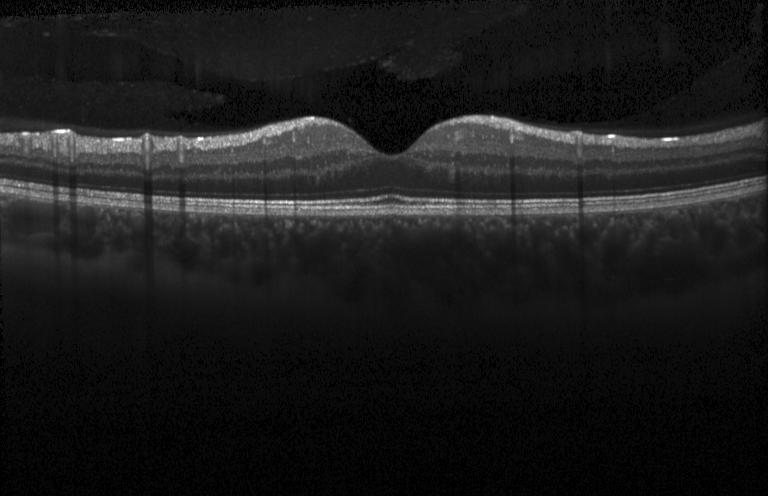 Spectral-domain optical coherence tomography · centered on the fovea · OCT line scan. The scan shows no evidence of CNV, DME, or drusen.